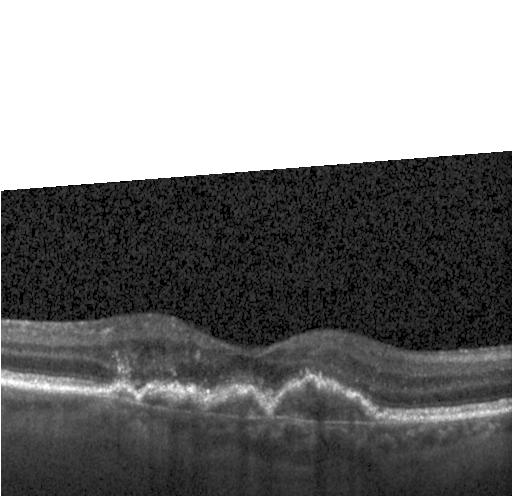

Macular OCT demonstrating choroidal neovascularization (CNV).